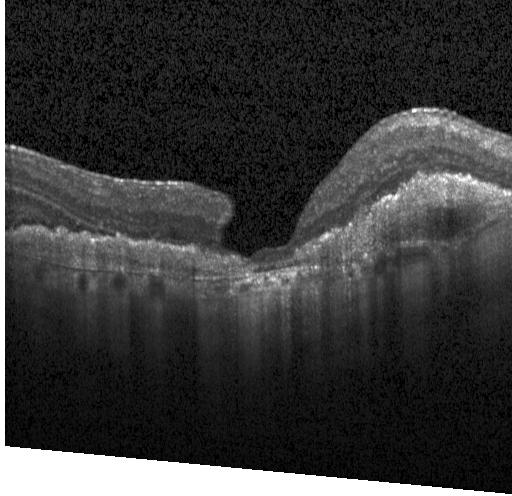 Retinal OCT B-scan; spectral-domain optical coherence tomography; centered on the fovea; acquired on a Heidelberg Spectralis.
Assessment: a choroidal neovascular membrane.